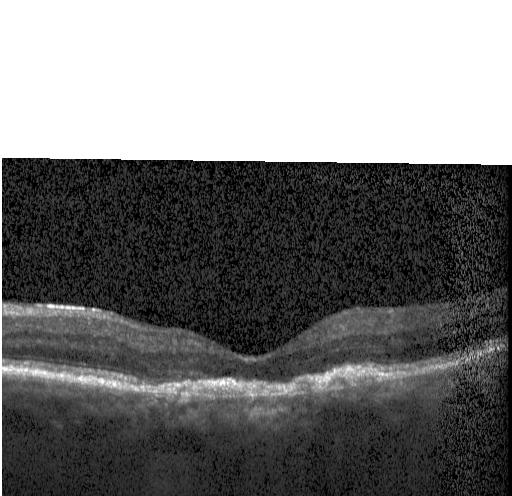
Heidelberg Spectralis OCT system. Spectral-domain OCT. Retinal OCT B-scan — Macular OCT: a choroidal neovascular membrane.